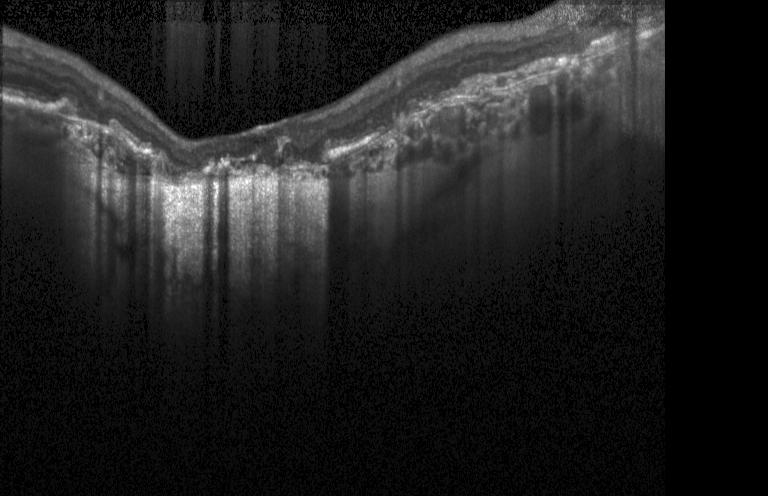 Optical coherence tomography B-scan; spectral-domain OCT; instrument: Heidelberg Spectralis.
Finding: a choroidal neovascular membrane.